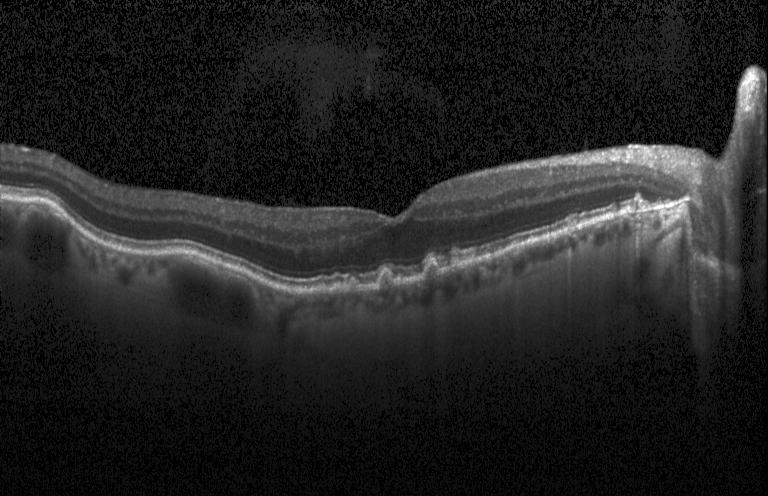

Spectral-domain OCT B-scan: drusen.